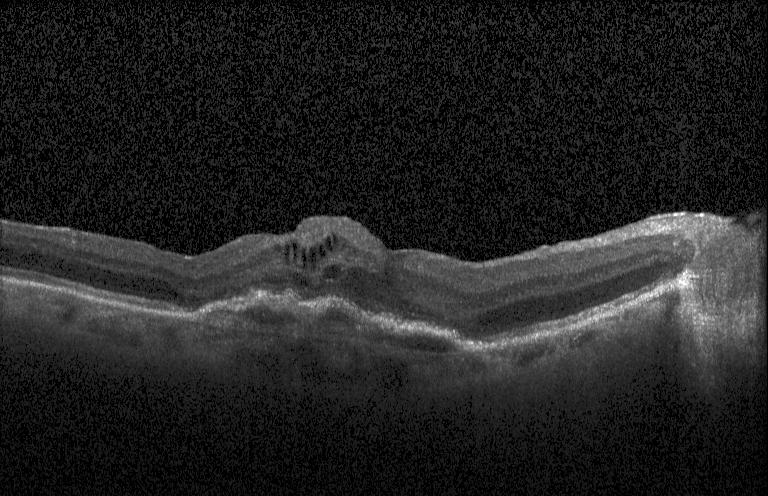
OCT line scan
Finding: a choroidal neovascular membrane.